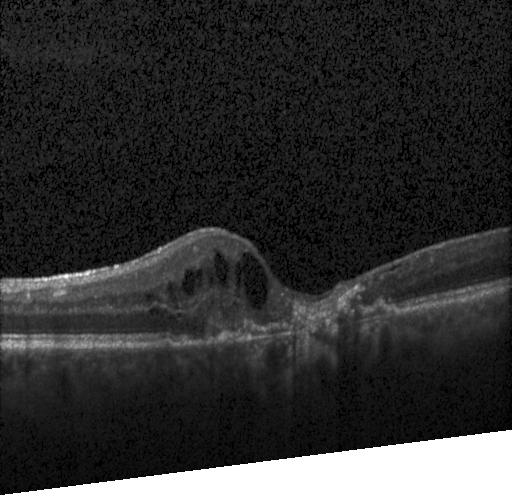
Retinal OCT cross-section. Spectral-domain OCT. Instrument: Heidelberg Spectralis. Centered on the fovea. The scan shows choroidal neovascularization (CNV).